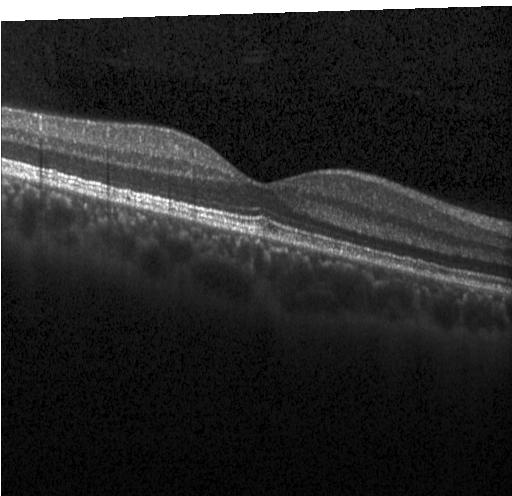

Assessment: no choroidal neovascularization, diabetic macular edema, or drusen.